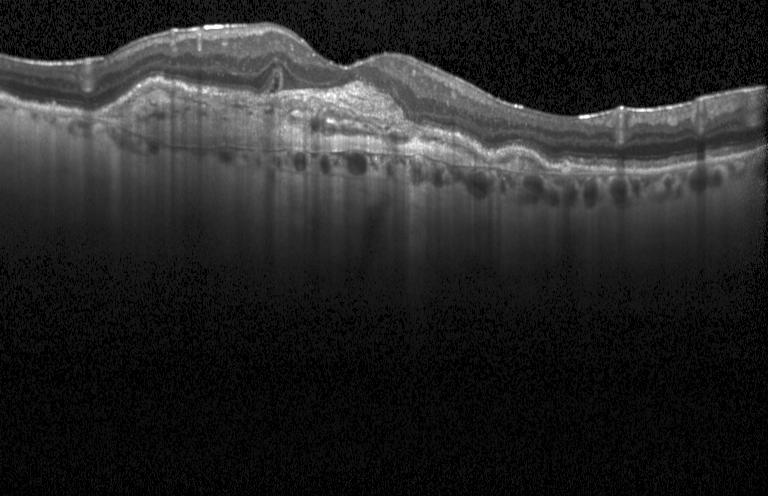

Spectral-domain optical coherence tomography · retinal OCT B-scan
Dx: choroidal neovascularization (CNV).